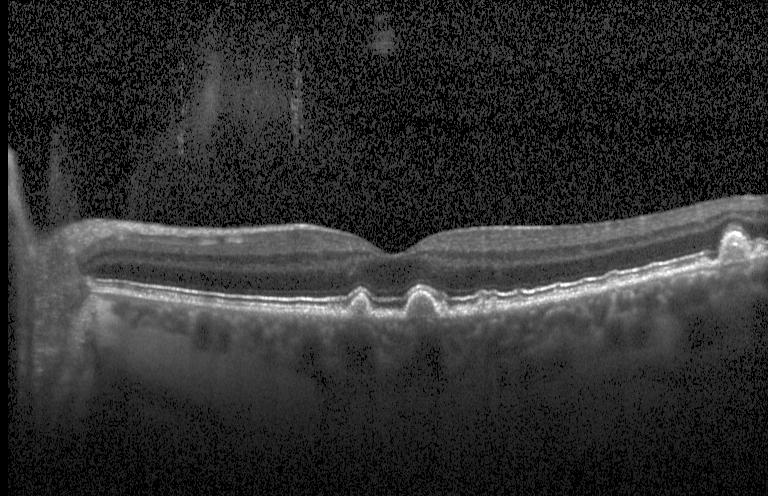
Finding: drusen.